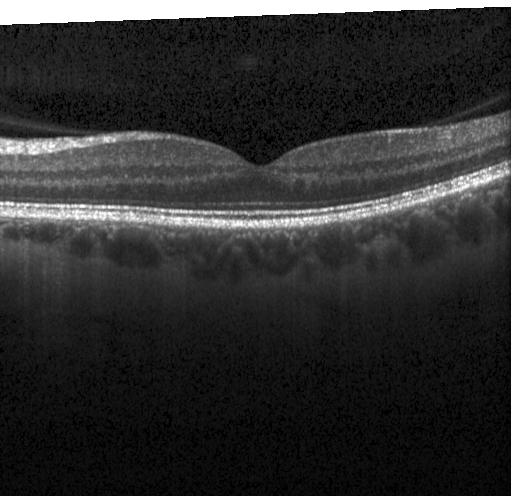

Centered on the fovea, SD-OCT, Heidelberg Spectralis OCT system, OCT B-scan.
OCT finding: neither choroidal neovascularization, diabetic macular edema, nor drusen.